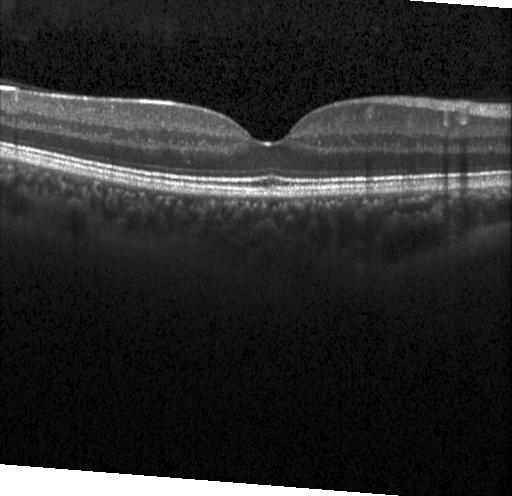

OCT line scan — Finding: no choroidal neovascularization, no diabetic macular edema, and no drusen.